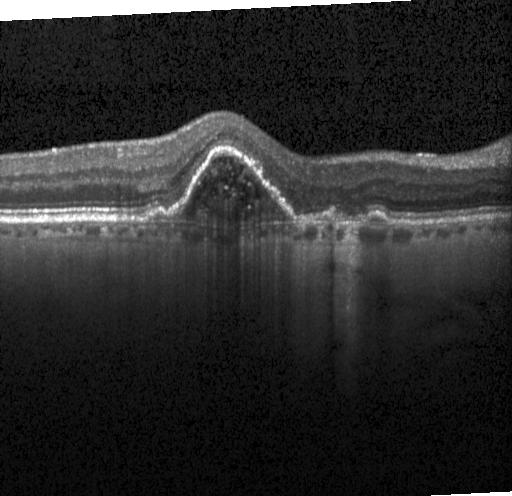 Spectral-domain OCT, Heidelberg Spectralis, centered on the fovea, retinal OCT cross-section.
Choroidal neovascularization.